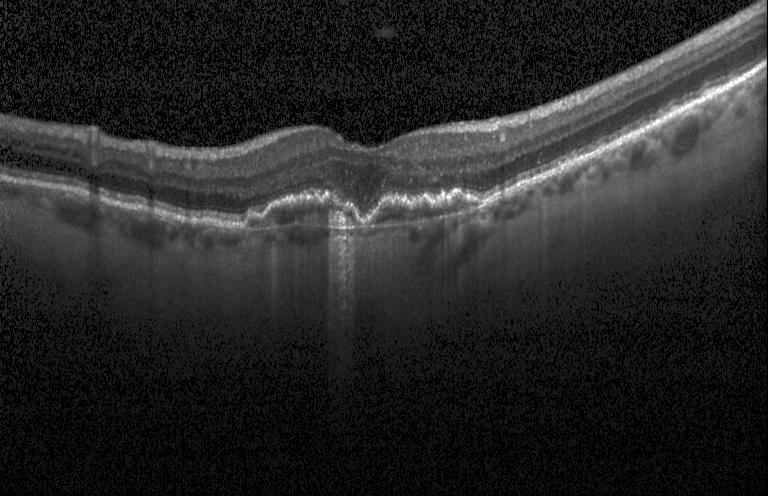

Optical coherence tomography B-scan. Finding: a choroidal neovascular membrane.